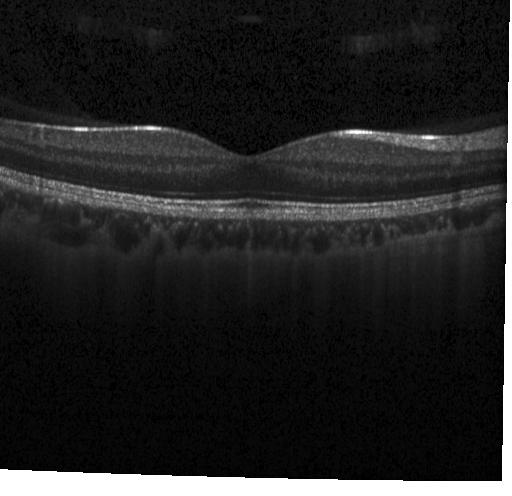
Macular scan; optical coherence tomography scan
No choroidal neovascularization, no diabetic macular edema, and no drusen.